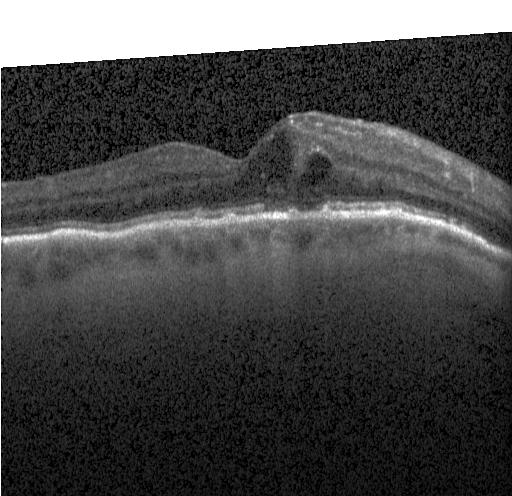

Spectral-domain optical coherence tomography. Acquired on a Heidelberg Spectralis. Optical coherence tomography B-scan. Macular OCT: DME.